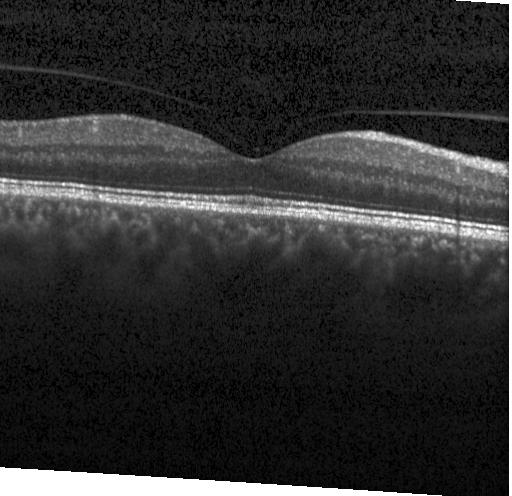
Heidelberg Spectralis; optical coherence tomography scan.
Impression: no choroidal neovascularization, no diabetic macular edema, and no drusen.